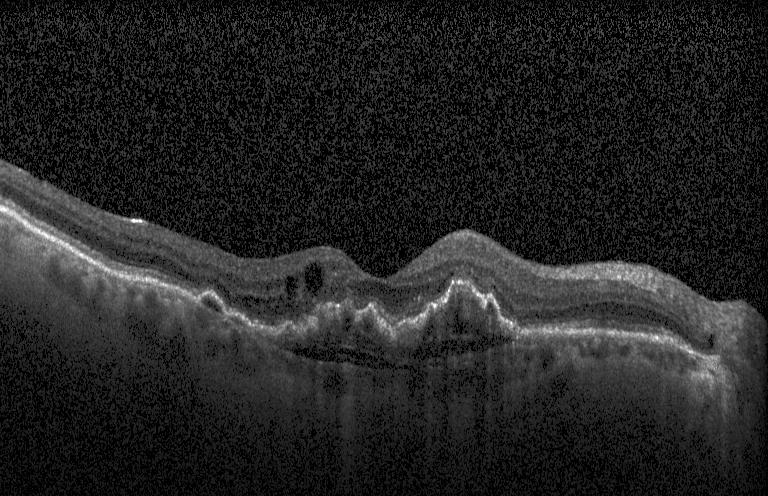
Macular OCT demonstrating CNV.